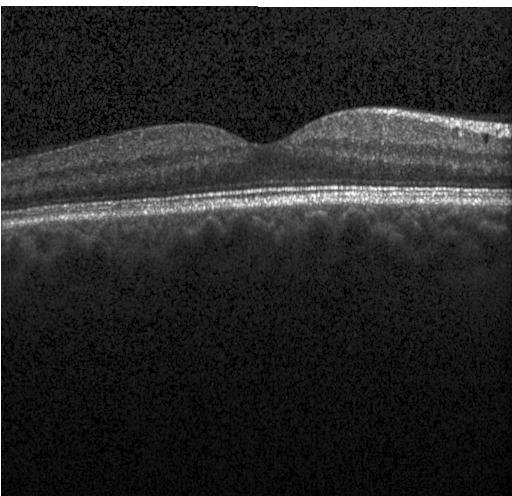 Impression: no CNV, DME, or drusen.